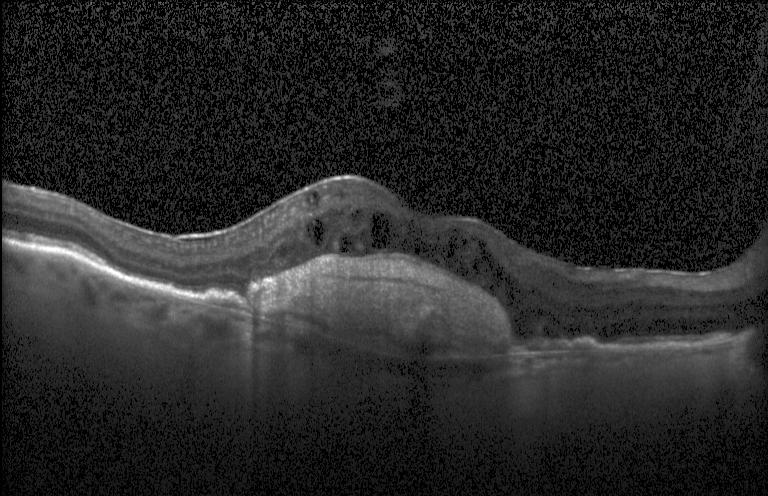

Centered on the fovea; retinal OCT cross-section; spectral-domain optical coherence tomography
Finding: choroidal neovascularization (CNV).